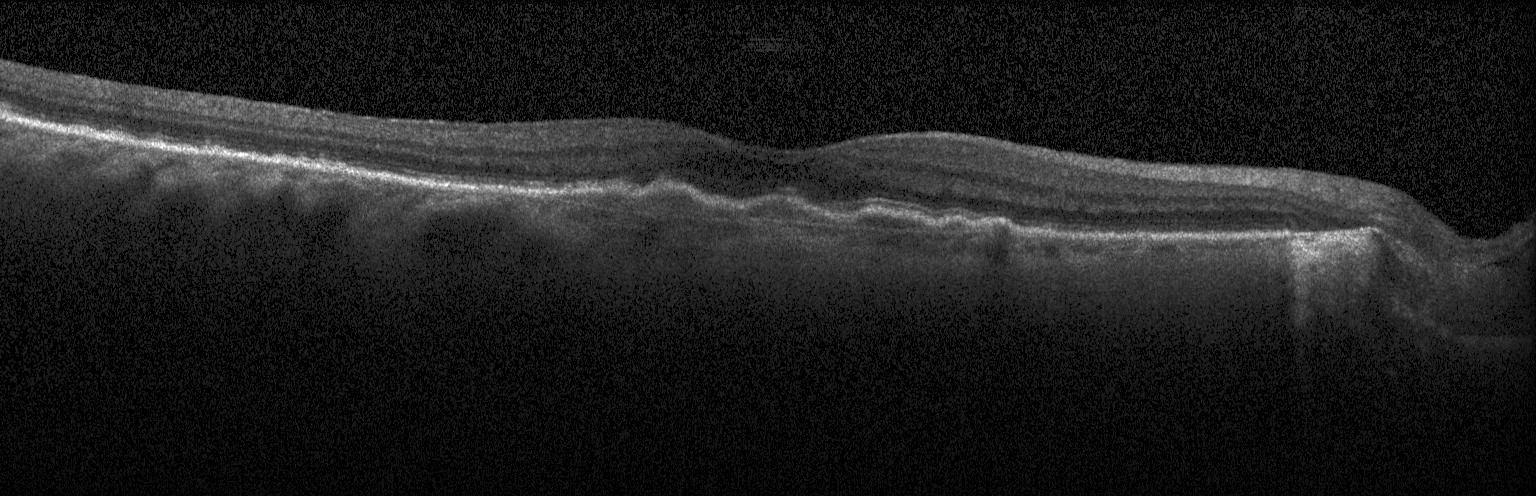
Diagnosis: a choroidal neovascular membrane.